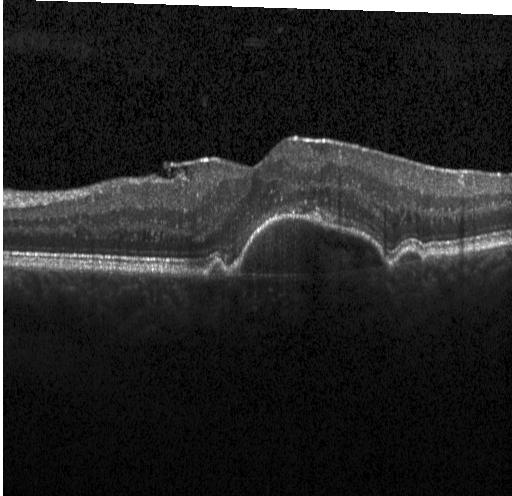 Impression: a choroidal neovascular membrane.